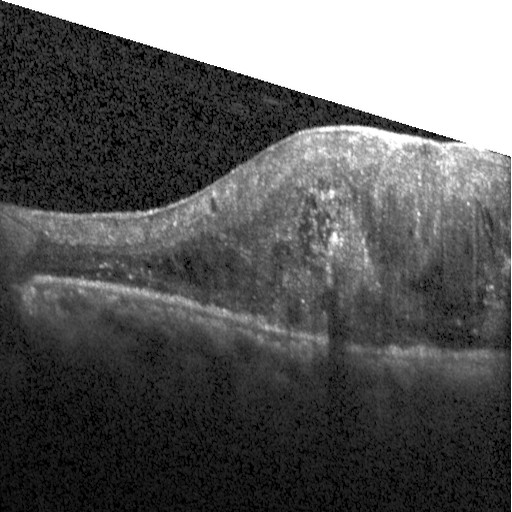 The scan shows diabetic macular edema.